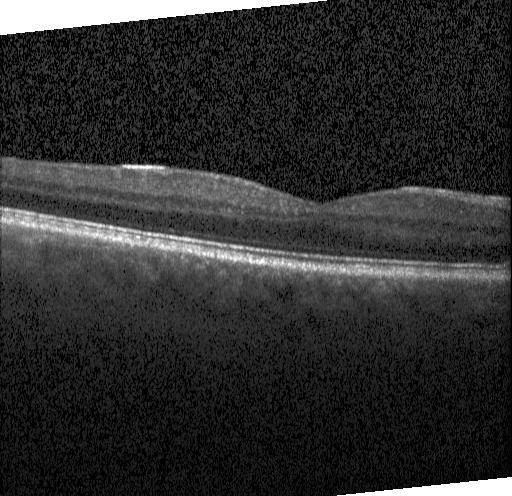 Optical coherence tomography B-scan.
Finding: no choroidal neovascularization, diabetic macular edema, or drusen.